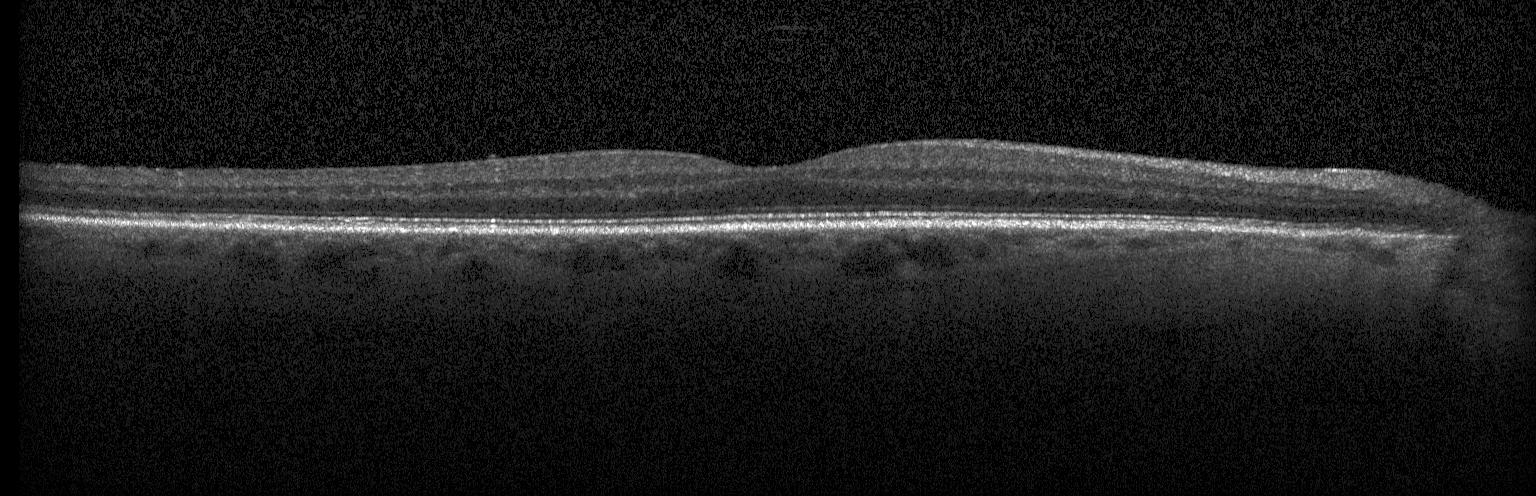

Spectral-domain optical coherence tomography. OCT B-scan. Heidelberg Spectralis OCT system.
Impression: no choroidal neovascularization, diabetic macular edema, or drusen.